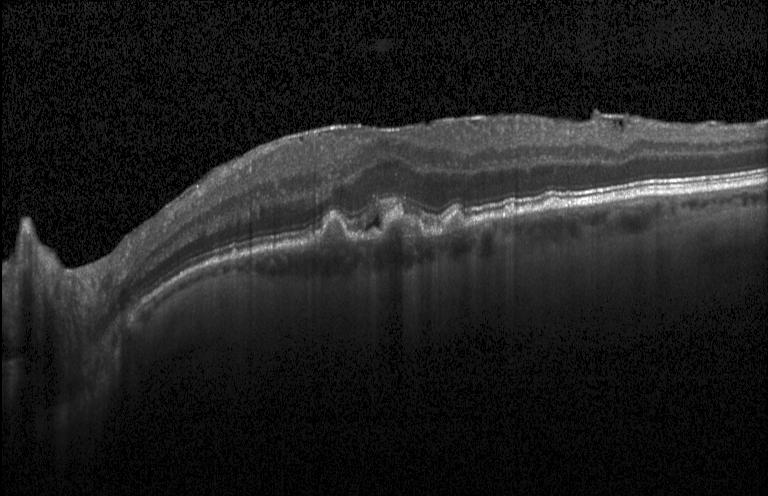

Optical coherence tomography scan · through the macula · SD-OCT · instrument: Heidelberg Spectralis.
Diagnosis: sub-RPE drusenoid deposits.